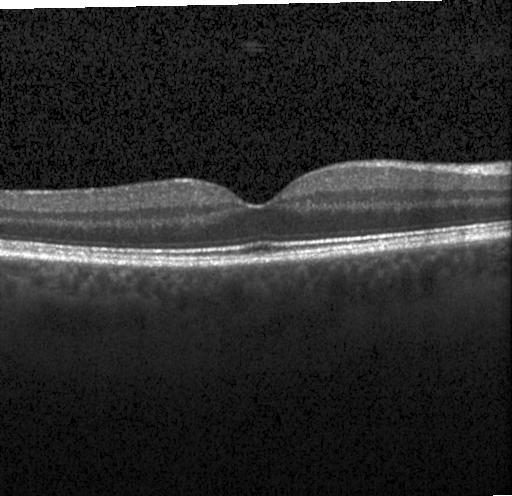 Impression: no choroidal neovascularization, diabetic macular edema, or drusen.